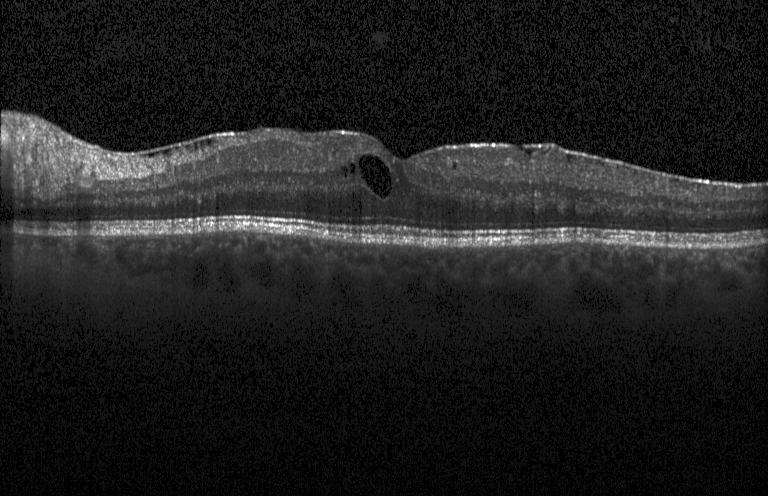
Macular scan; optical coherence tomography B-scan
Finding: DME.